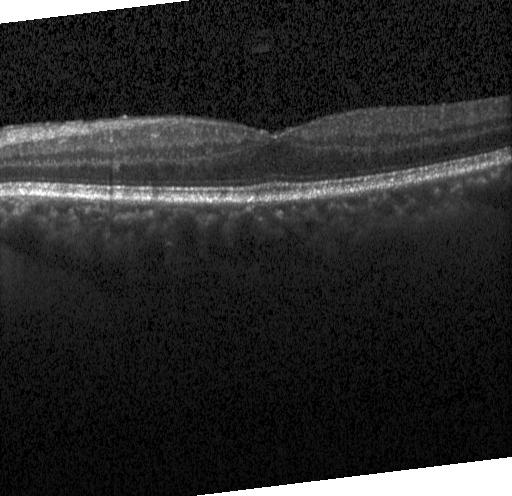
Acquired on a Heidelberg Spectralis. Spectral-domain optical coherence tomography. Retinal OCT cross-section.
Diagnosis: neither CNV, DME, nor drusen.